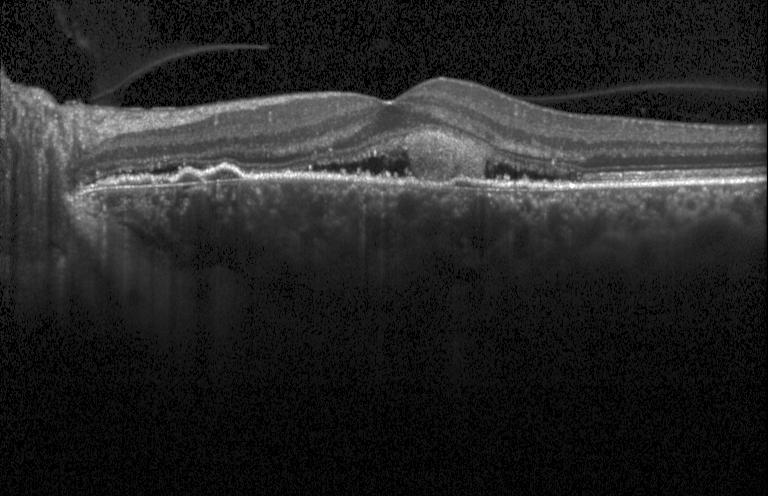
OCT line scan.
Finding: choroidal neovascularization.